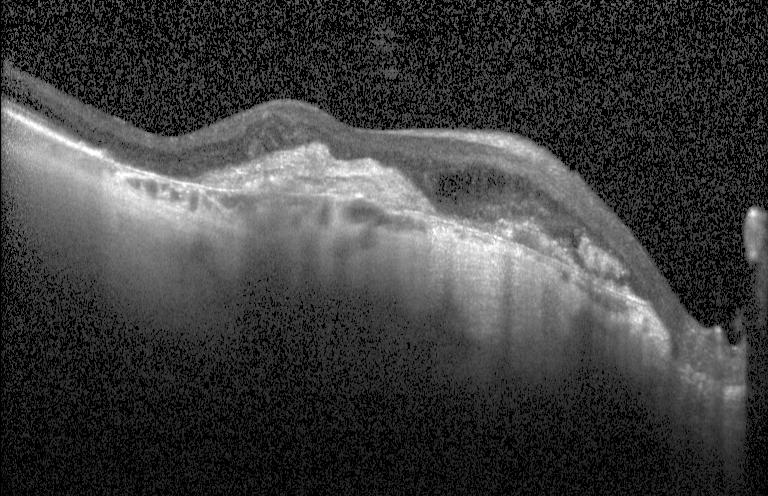

Diagnosis: a choroidal neovascular membrane.